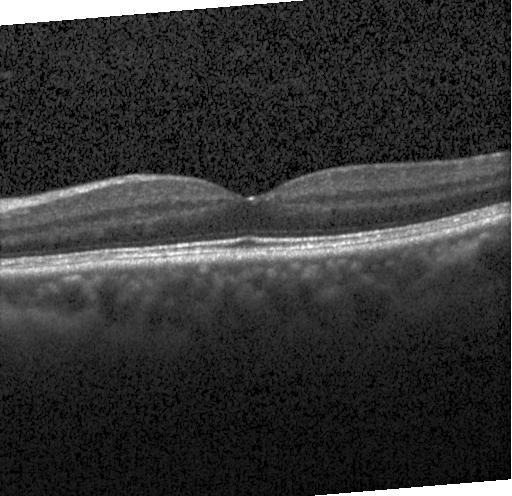 OCT scan showing neither choroidal neovascularization, diabetic macular edema, nor drusen.